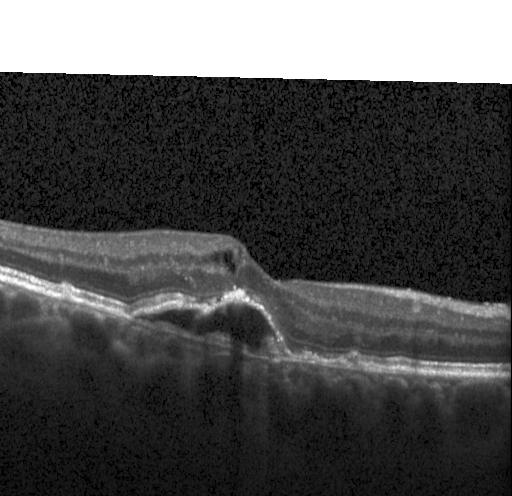 Spectral-domain optical coherence tomography · OCT line scan. Finding: CNV.